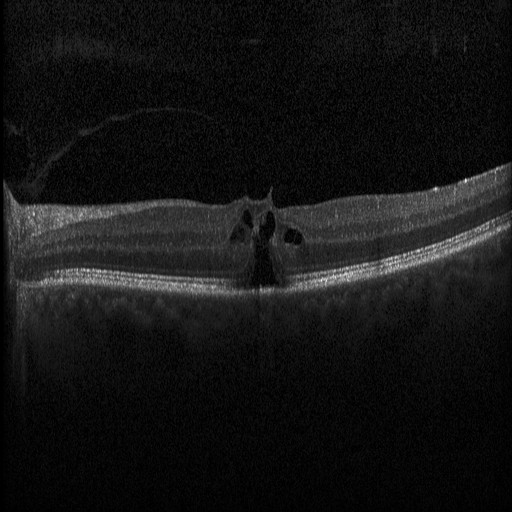

Spectral-domain optical coherence tomography. Horizontal scan through the fovea. Optical coherence tomography B-scan.
Diabetic macular edema.